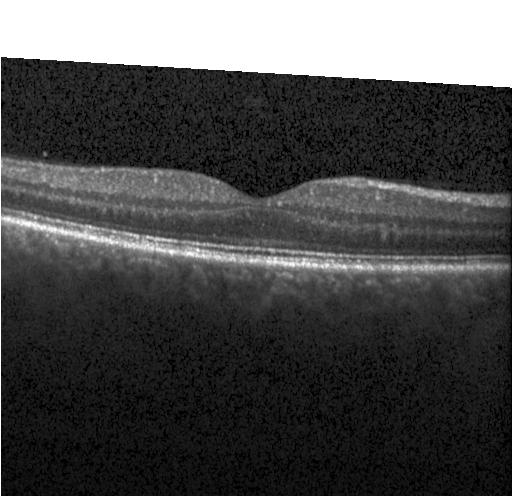 Acquired on a Heidelberg Spectralis, spectral-domain OCT, retinal OCT cross-section, centered on the fovea
The scan shows neither CNV, DME, nor drusen.